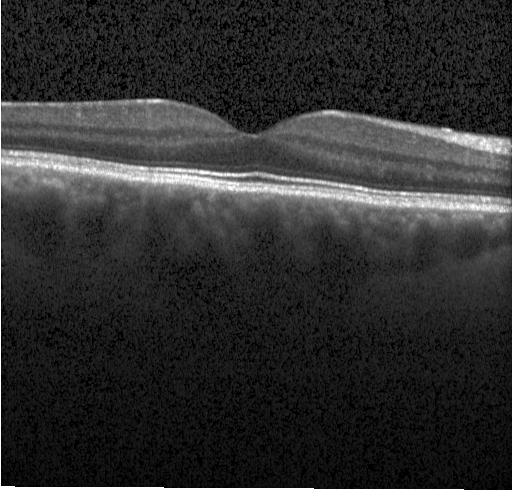

Heidelberg Spectralis, spectral-domain optical coherence tomography, OCT B-scan, macular scan — This B-scan demonstrates no evidence of CNV, DME, or drusen.